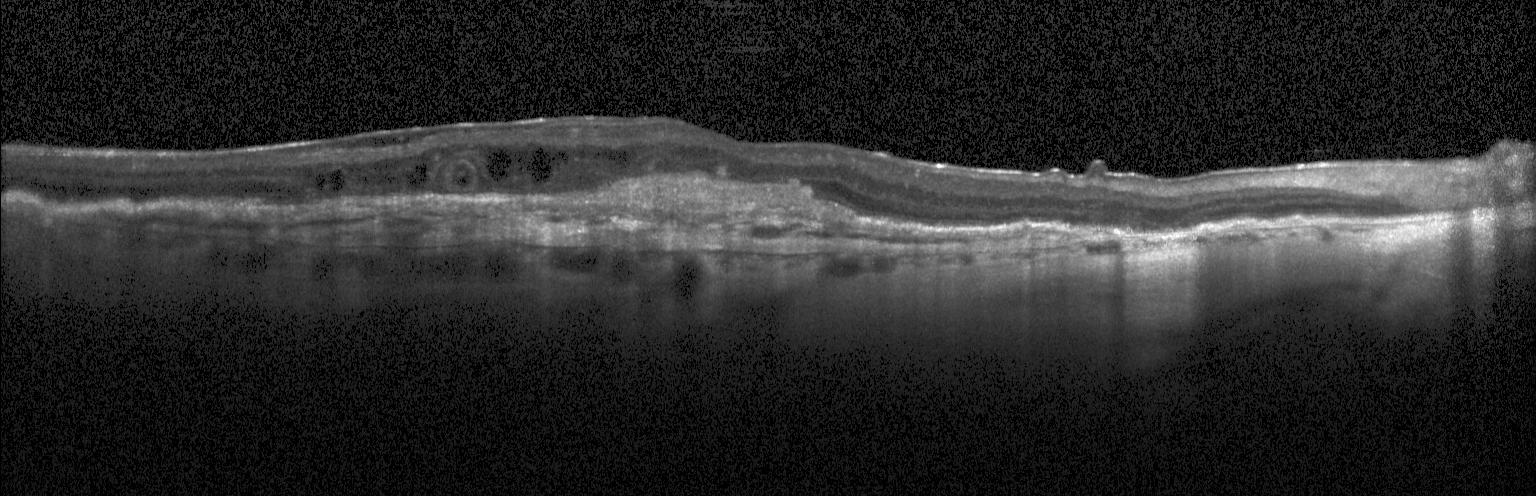
Impression: a choroidal neovascular membrane.